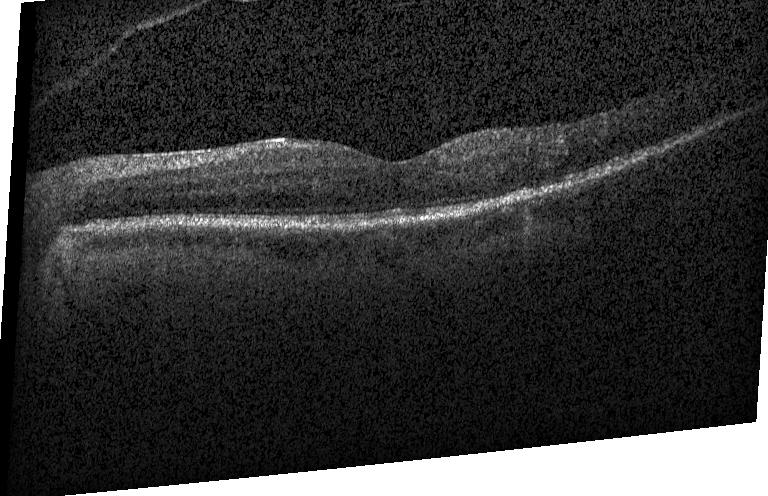 OCT line scan — Diagnosis: DME.